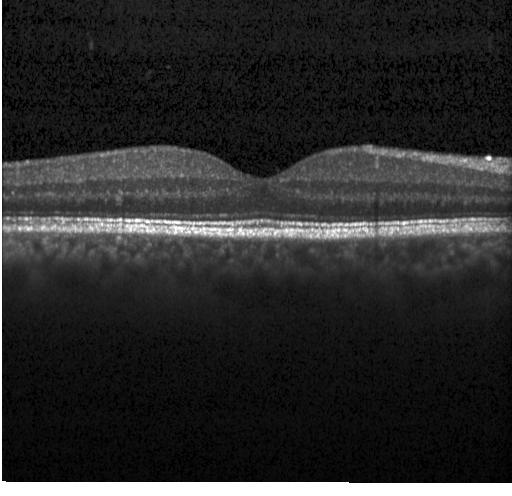
OCT finding: no evidence of choroidal neovascularization, diabetic macular edema, or drusen.